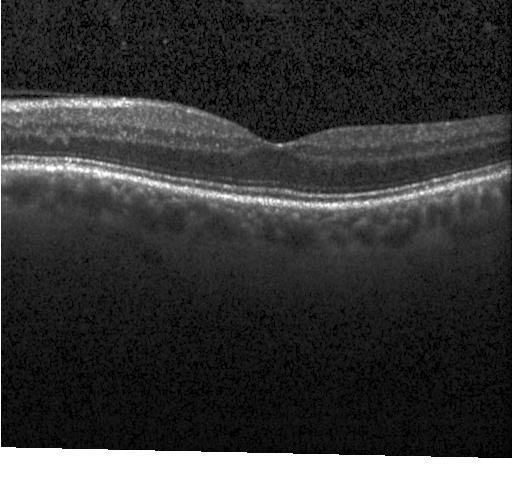

Optical coherence tomography B-scan, spectral-domain OCT, acquired on a Heidelberg Spectralis. Finding: neither CNV, DME, nor drusen.